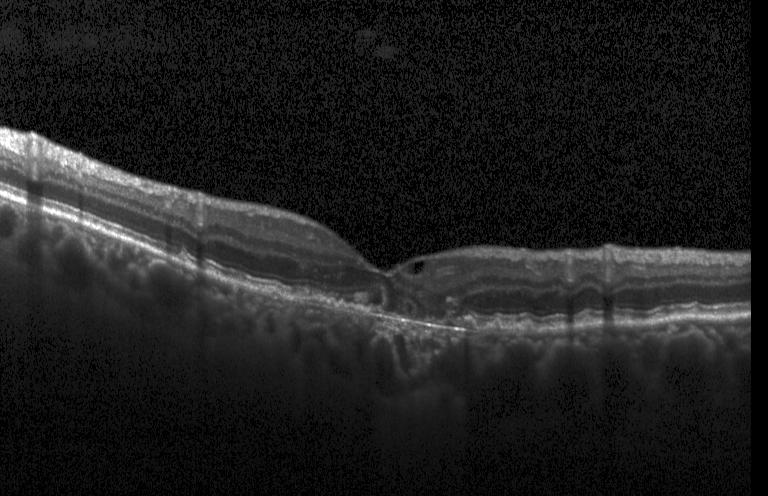
Instrument: Heidelberg Spectralis, retinal OCT B-scan, SD-OCT.
Impression: a choroidal neovascular membrane.